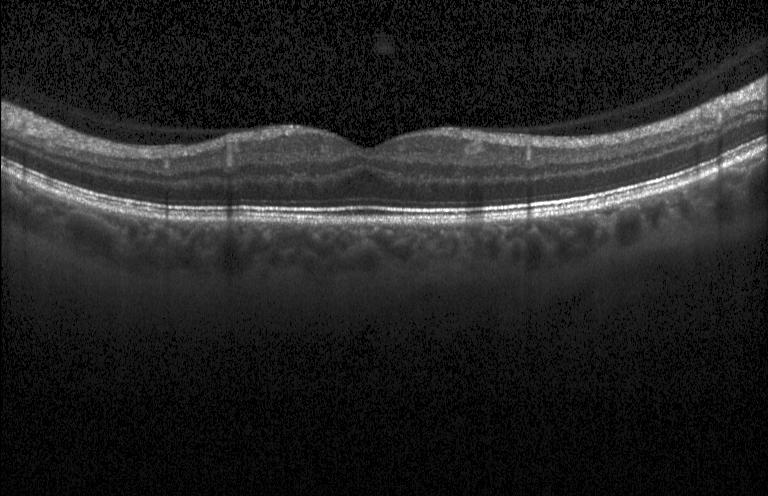

SD-OCT; macular scan; optical coherence tomography B-scan. Assessment: no evidence of choroidal neovascularization, diabetic macular edema, or drusen.